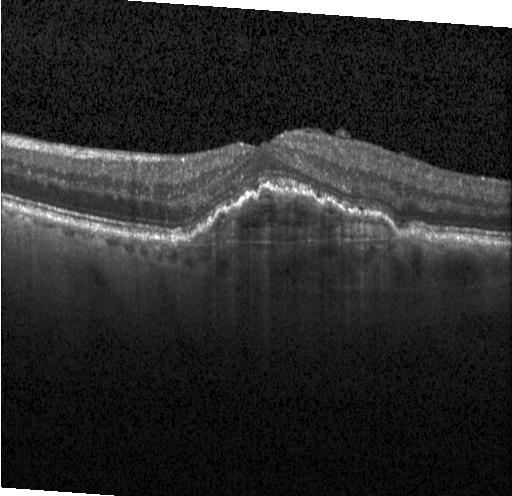 Macular OCT demonstrating a choroidal neovascular membrane.